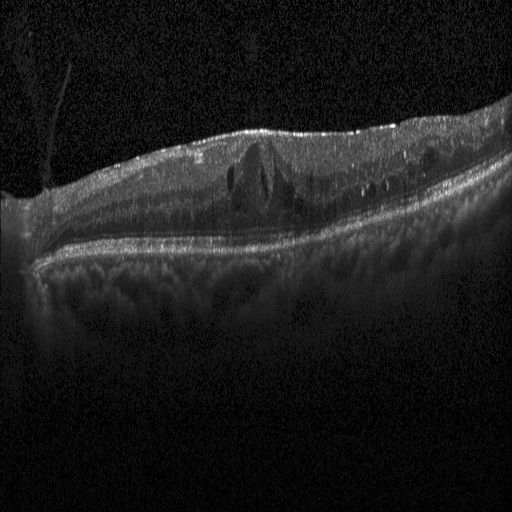
Instrument: Heidelberg Spectralis; optical coherence tomography B-scan; spectral-domain optical coherence tomography; through the macula — The scan shows diabetic macular edema.